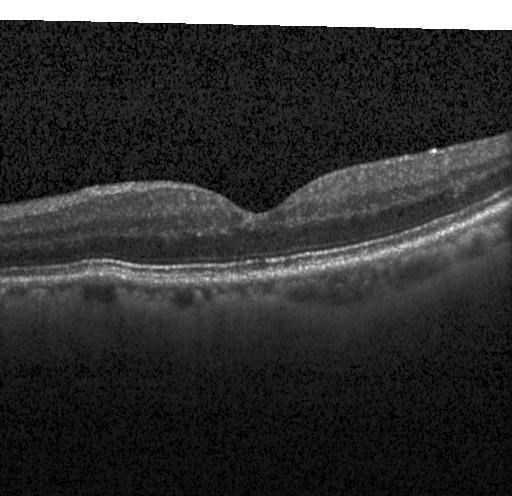
OCT B-scan showing no choroidal neovascularization, no diabetic macular edema, and no drusen.